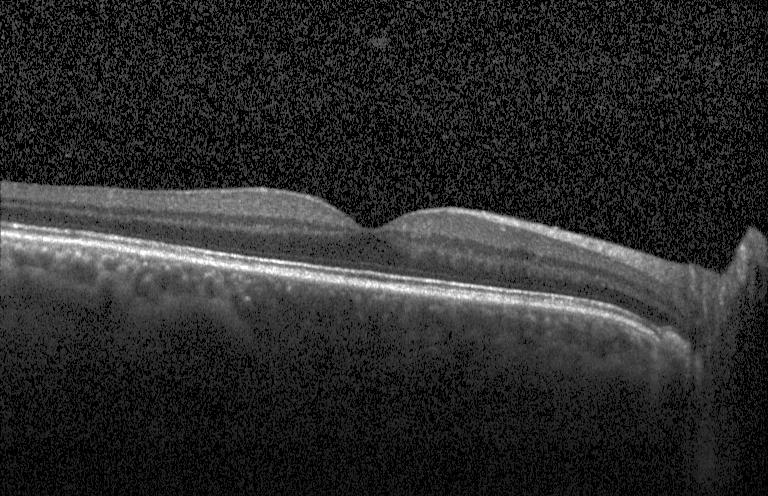
OCT scan showing no CNV, no DME, and no drusen.